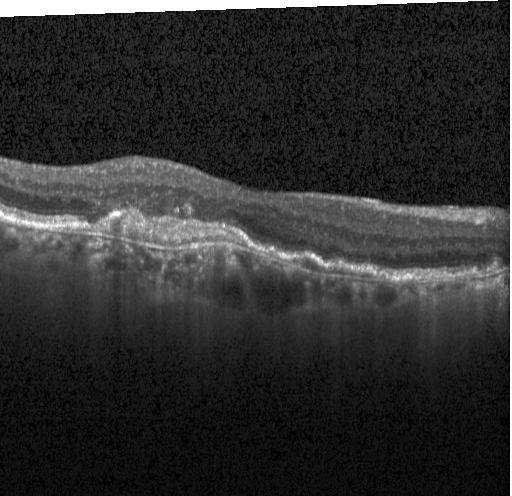
Spectral-domain OCT B-scan: choroidal neovascularization (CNV).